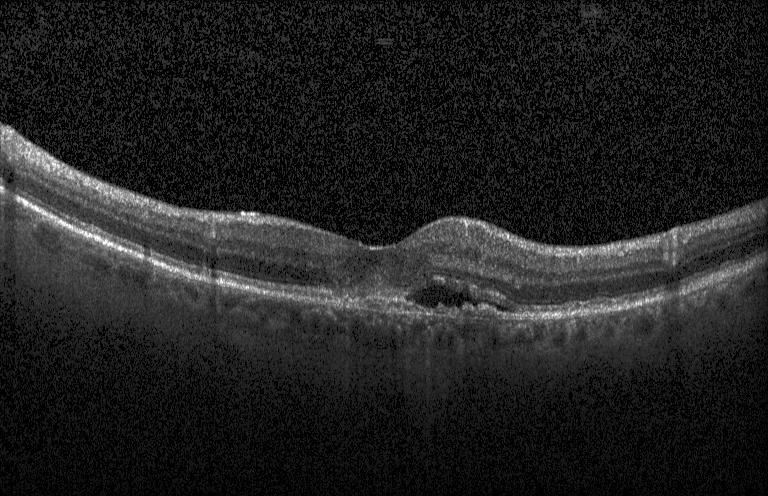

Instrument: Heidelberg Spectralis. Optical coherence tomography scan. OCT finding: a choroidal neovascular membrane.